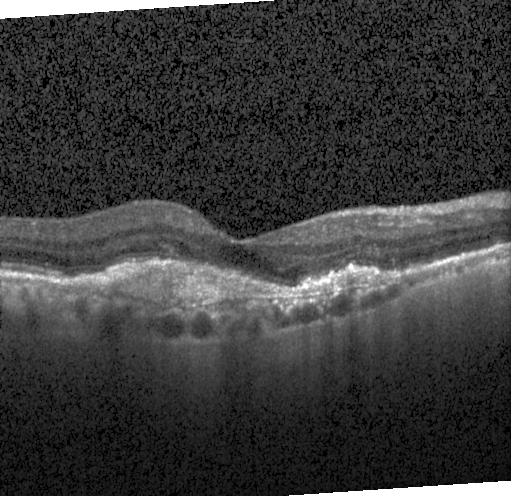 Finding: choroidal neovascularization.